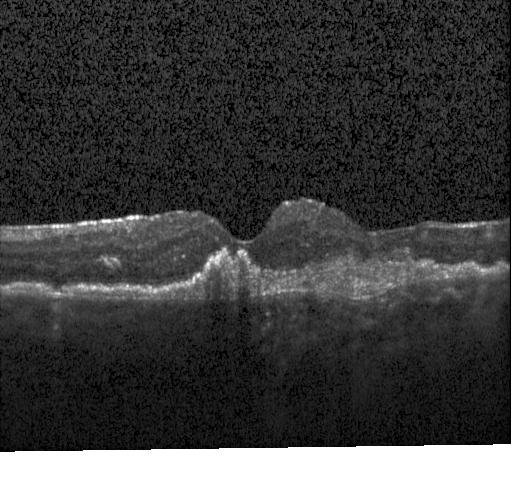
This B-scan demonstrates CNV.